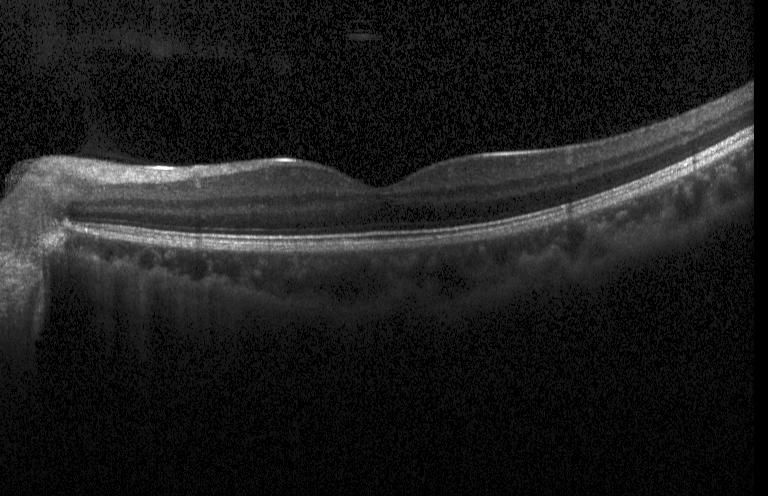
OCT B-scan; spectral-domain OCT; through the macula — This B-scan demonstrates neither choroidal neovascularization, diabetic macular edema, nor drusen.